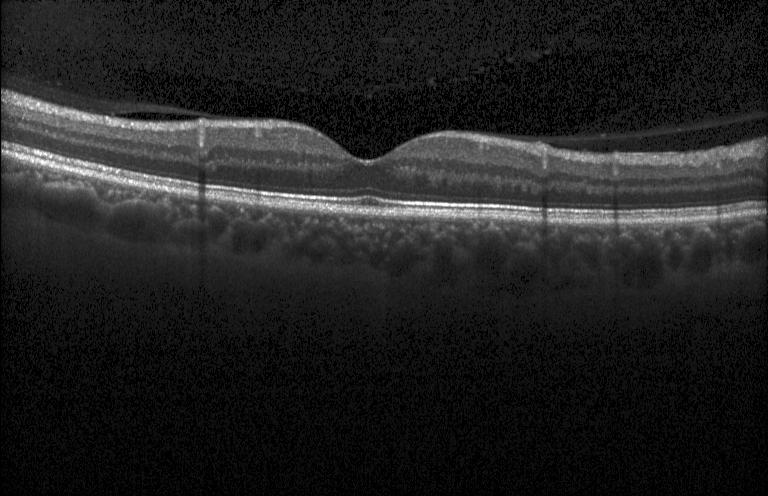 Diagnosis: neither choroidal neovascularization, diabetic macular edema, nor drusen.